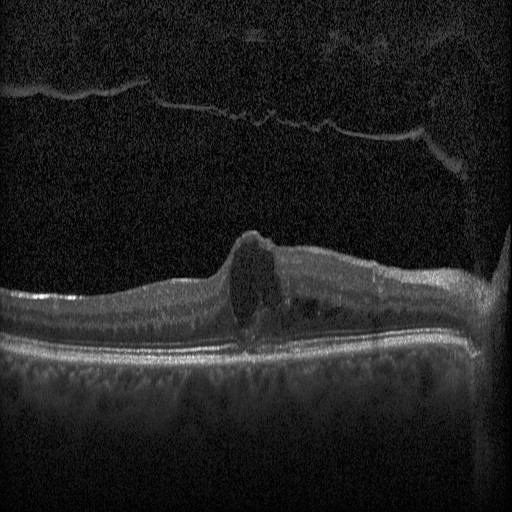

Retinal OCT cross-section showing diabetic macular edema.